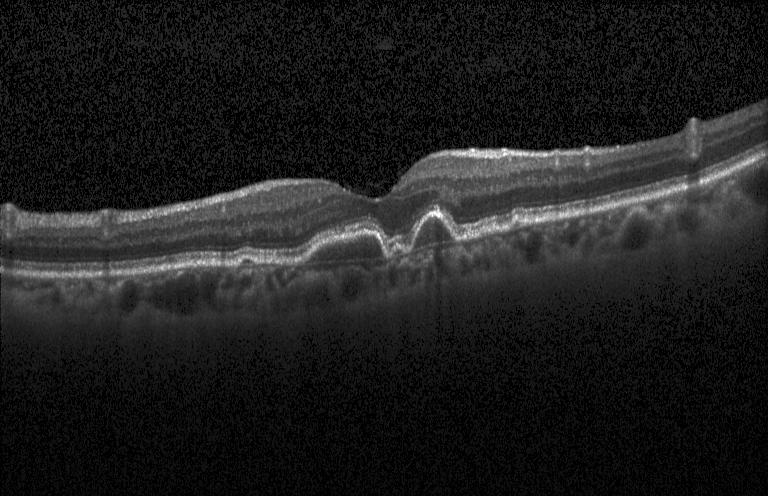 Diagnosis: a choroidal neovascular membrane.